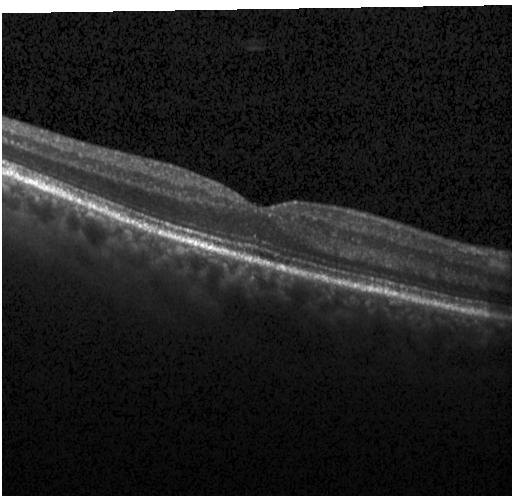

OCT line scan — Impression: neither CNV, DME, nor drusen.